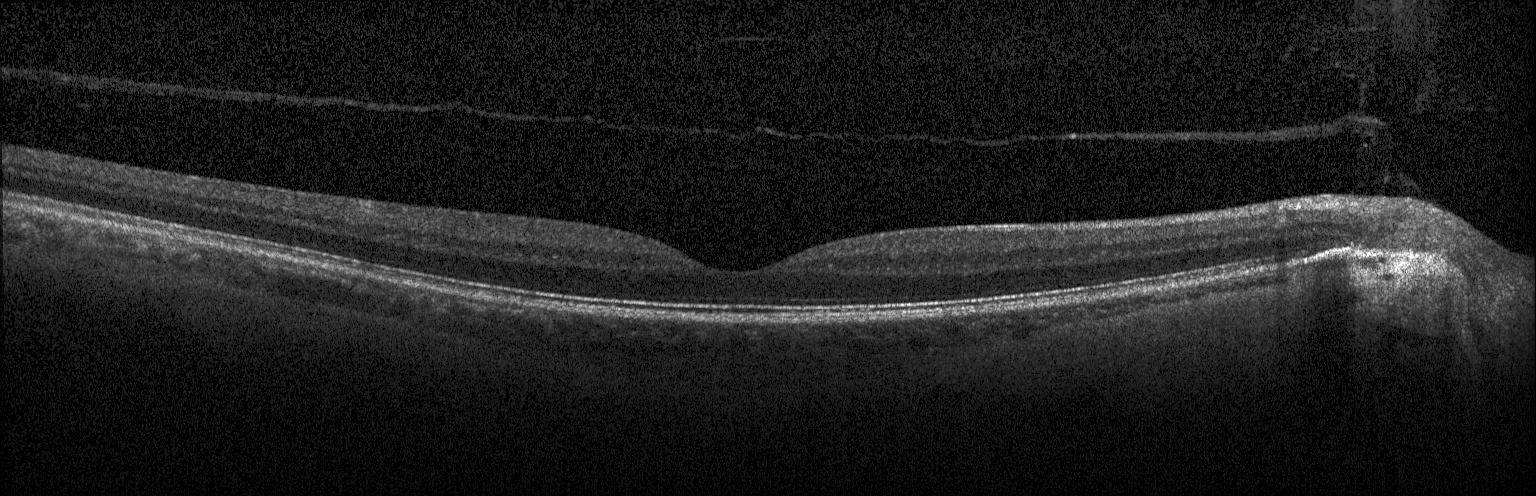
OCT B-scan showing no CNV, no DME, and no drusen.